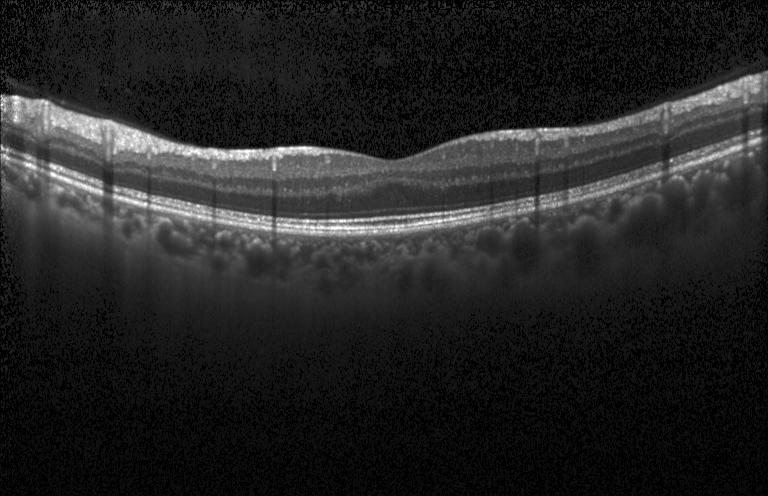
Retinal OCT B-scan. The scan shows no CNV, DME, or drusen.